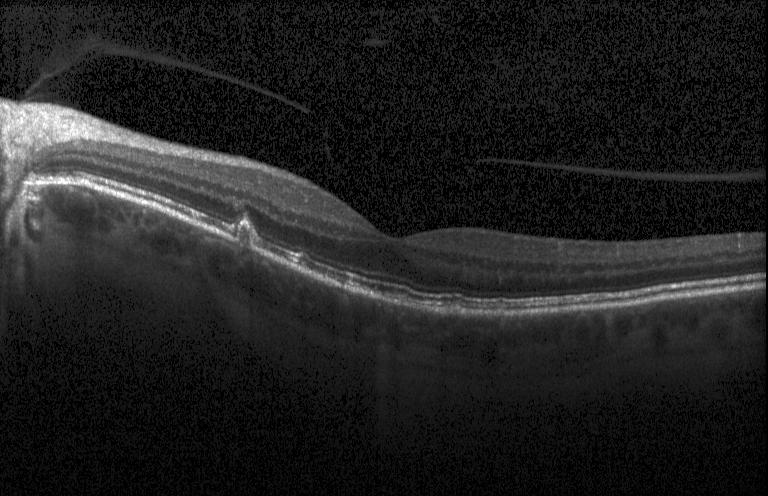
Horizontal scan through the fovea; OCT line scan — This B-scan demonstrates multiple drusen.